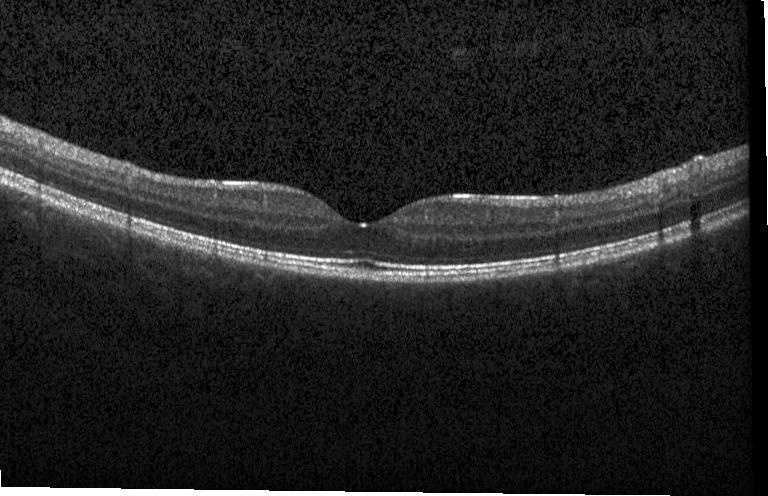 Macular scan; SD-OCT; Heidelberg Spectralis; OCT line scan
Diagnosis: no CNV, no DME, and no drusen.